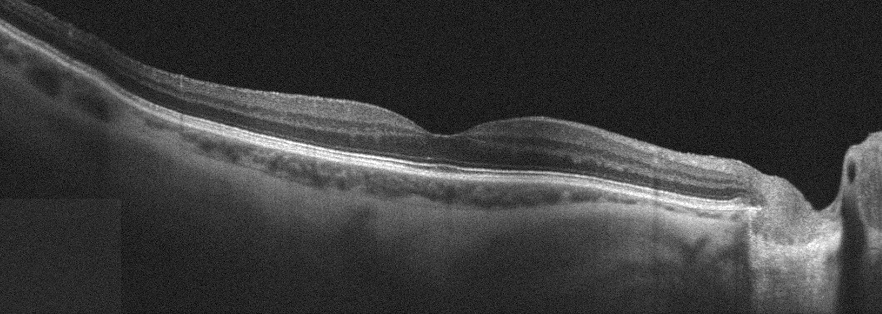
OCT B-scan, fovea-centered.
Assessment: no AMD, DME, ERM, RAO, RVO, or VID.